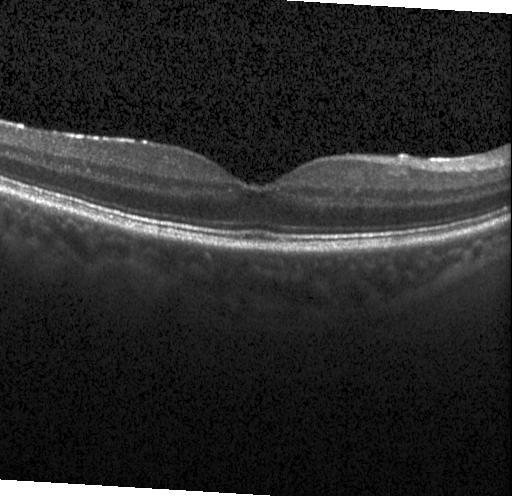
Finding: no choroidal neovascularization, no diabetic macular edema, and no drusen.